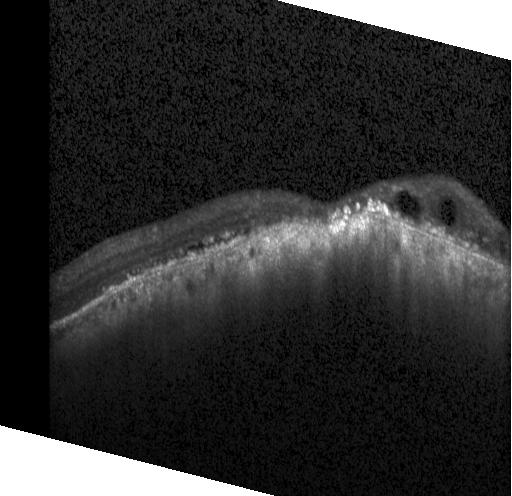 Centered on the fovea. Retinal OCT cross-section. Spectral-domain optical coherence tomography.
Finding: choroidal neovascularization.